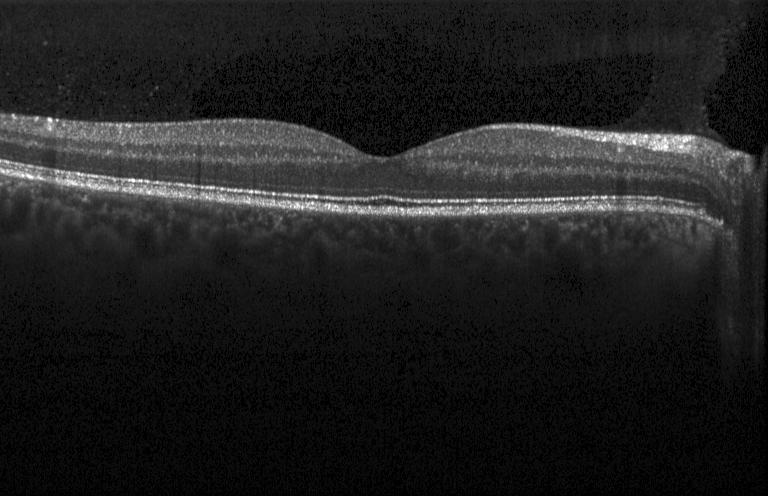

Retinal OCT cross-section. Spectral-domain optical coherence tomography — Assessment: no evidence of choroidal neovascularization, diabetic macular edema, or drusen.